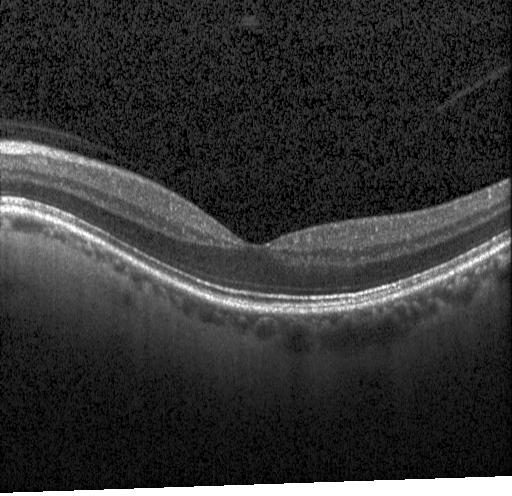
Diagnosis: neither CNV, DME, nor drusen.